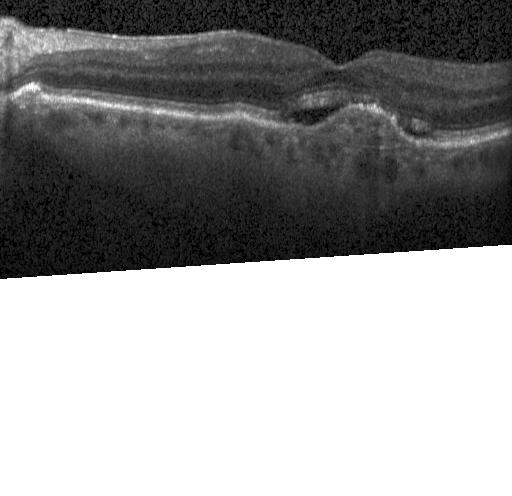

Horizontal scan through the fovea; spectral-domain OCT; retinal OCT cross-section.
Diagnosis: a choroidal neovascular membrane.